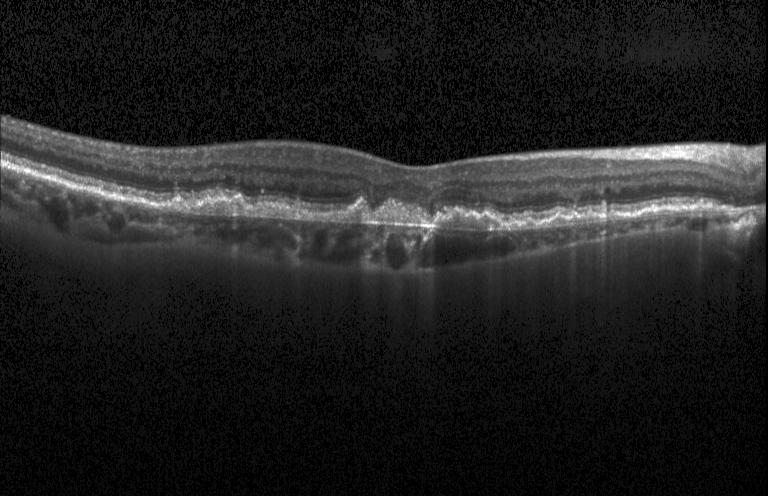 OCT B-scan
Finding: a choroidal neovascular membrane.